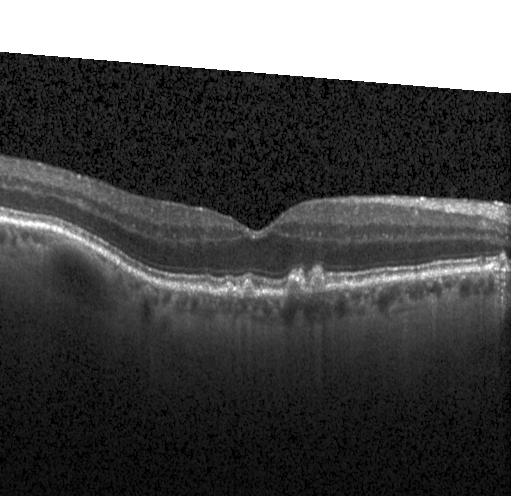 Acquired on a Heidelberg Spectralis, retinal OCT B-scan. Assessment: drusen.